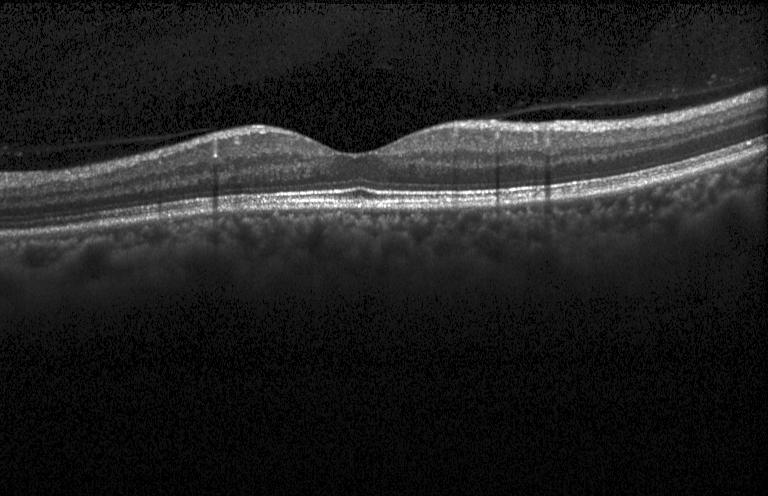

Retinal OCT B-scan. Diagnosis: no choroidal neovascularization, no diabetic macular edema, and no drusen.